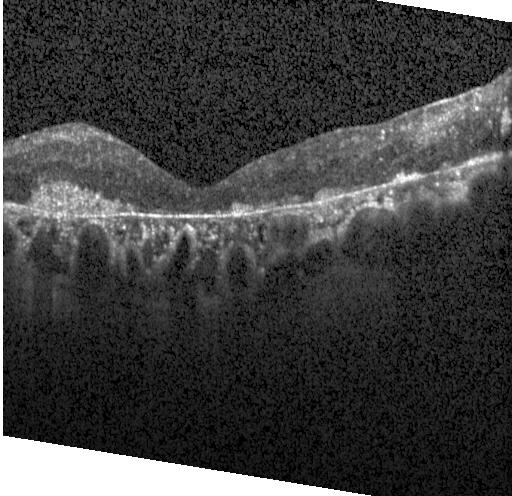
SD-OCT, fovea-centered, OCT line scan, instrument: Heidelberg Spectralis.
Finding: a choroidal neovascular membrane.